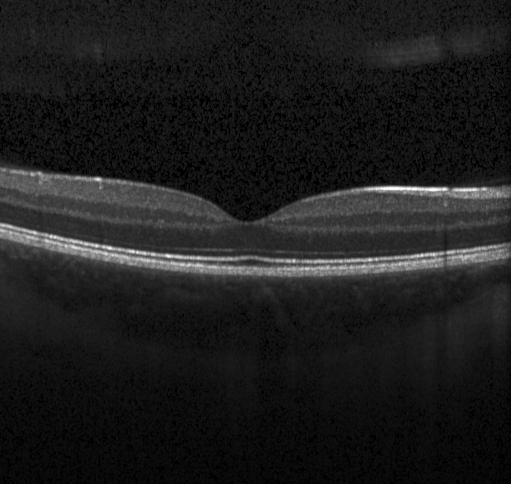

Heidelberg Spectralis · retinal OCT B-scan · SD-OCT · centered on the fovea — Diagnosis: neither choroidal neovascularization, diabetic macular edema, nor drusen.